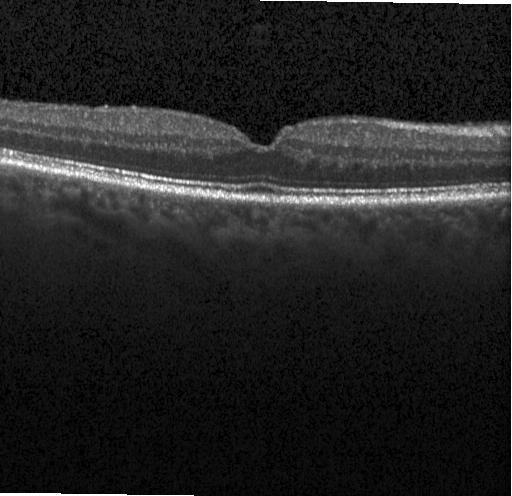 Spectral-domain OCT, centered on the fovea, instrument: Heidelberg Spectralis, retinal OCT B-scan. Finding: neither choroidal neovascularization, diabetic macular edema, nor drusen.